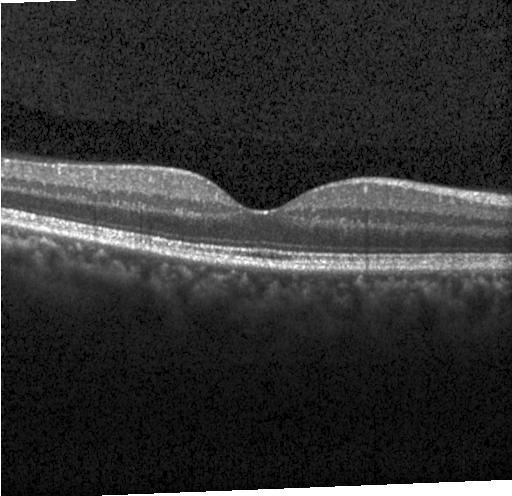 Spectral-domain OCT B-scan: no choroidal neovascularization, diabetic macular edema, or drusen.